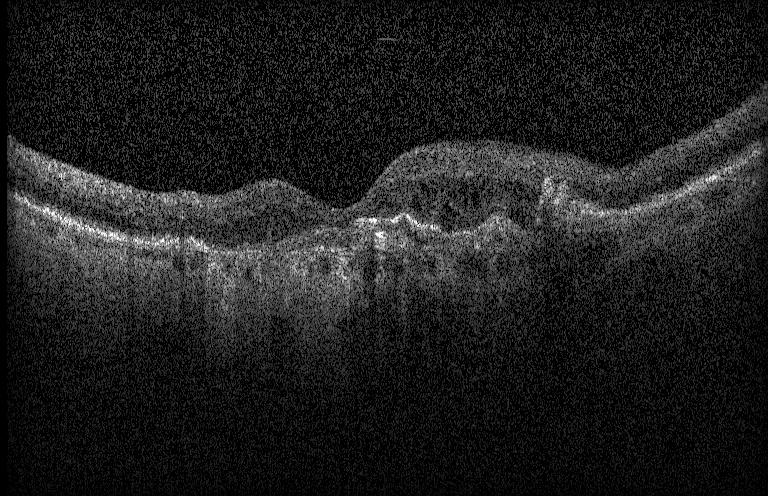
Spectral-domain optical coherence tomography; OCT line scan.
Macular OCT: a choroidal neovascular membrane.